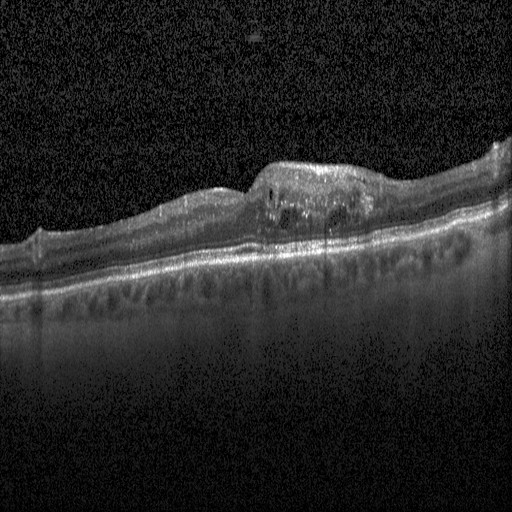 Macular OCT demonstrating diabetic macular edema.